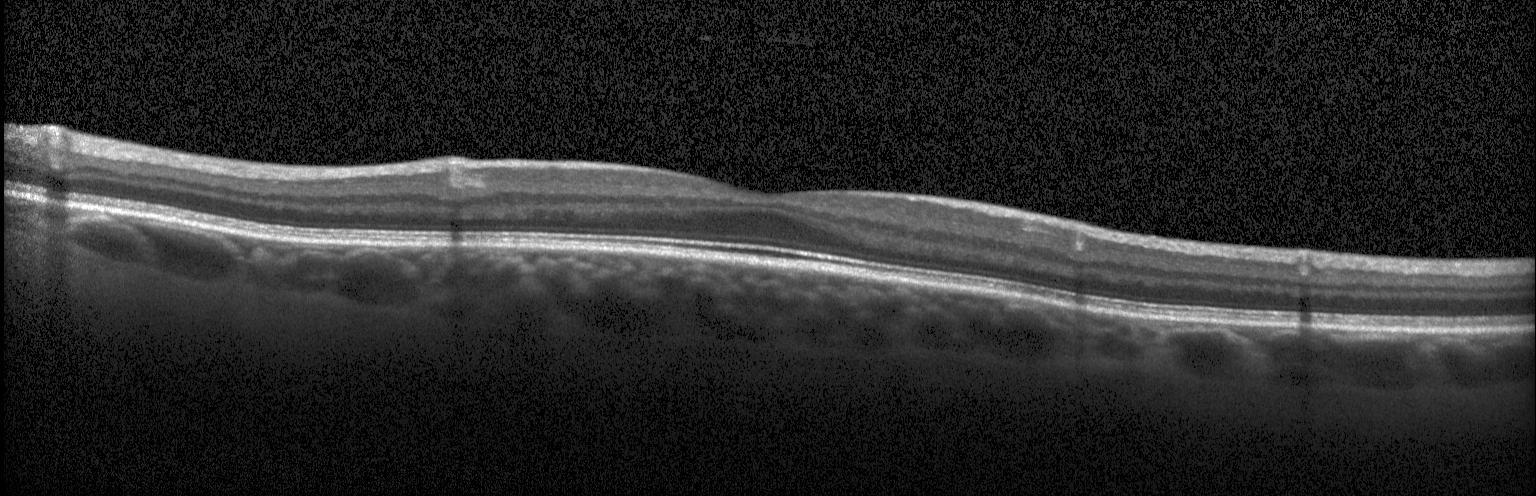
Finding: no CNV, no DME, and no drusen.